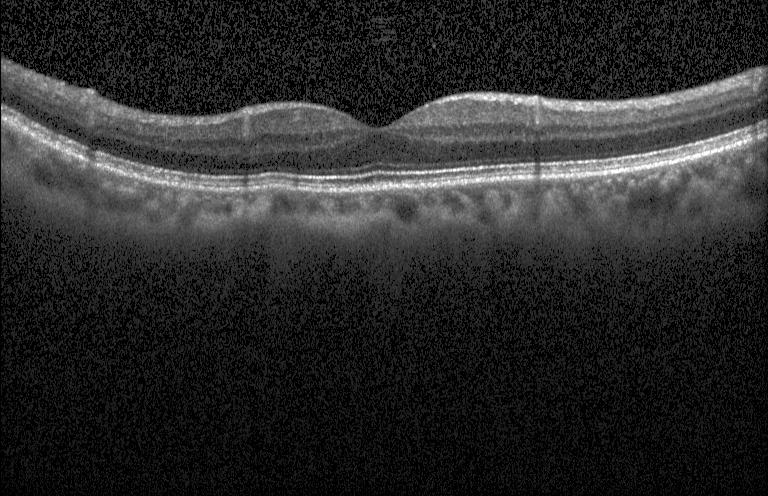

Heidelberg Spectralis. Retinal OCT B-scan. Centered on the fovea. Assessment: no CNV, DME, or drusen.